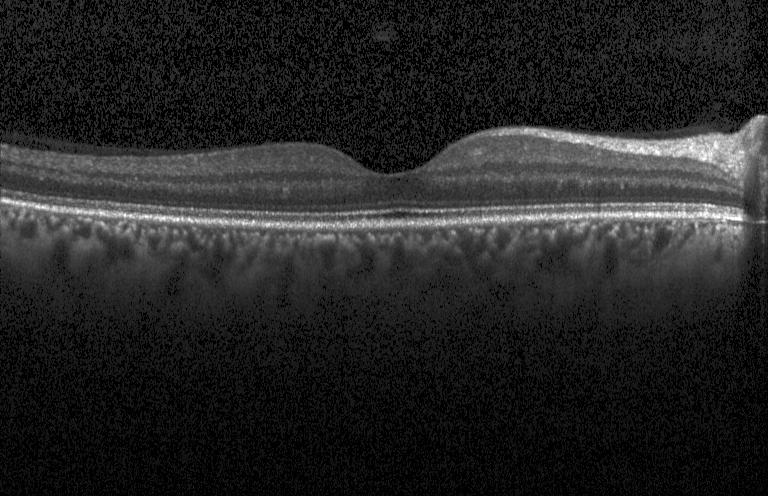

Finding: no choroidal neovascularization, diabetic macular edema, or drusen.